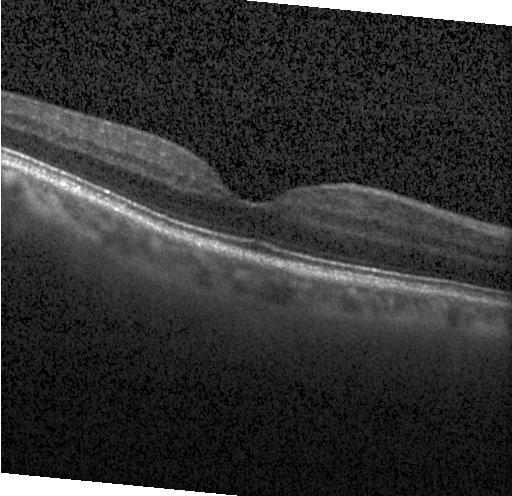

Retinal OCT cross-section
No evidence of choroidal neovascularization, diabetic macular edema, or drusen.